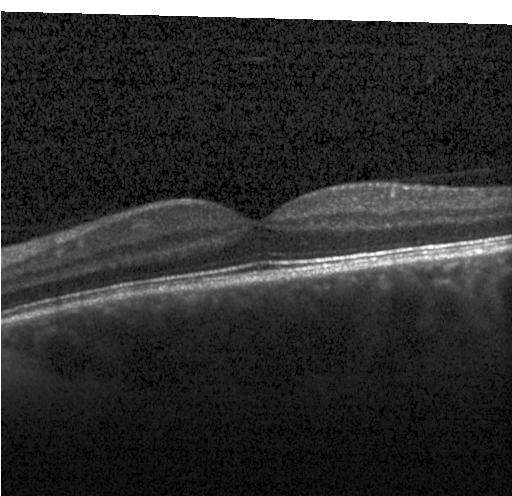
No CNV, DME, or drusen.